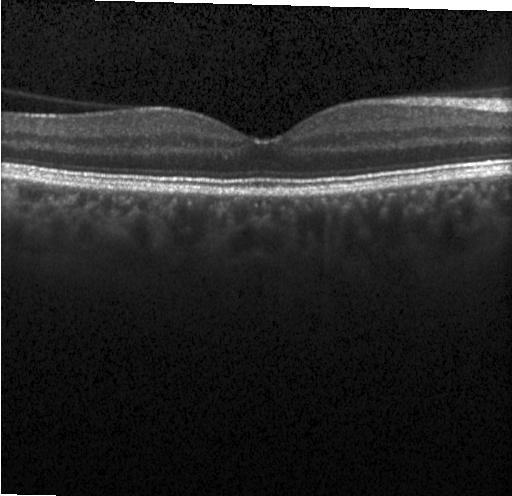
Macular OCT demonstrating no choroidal neovascularization, no diabetic macular edema, and no drusen.